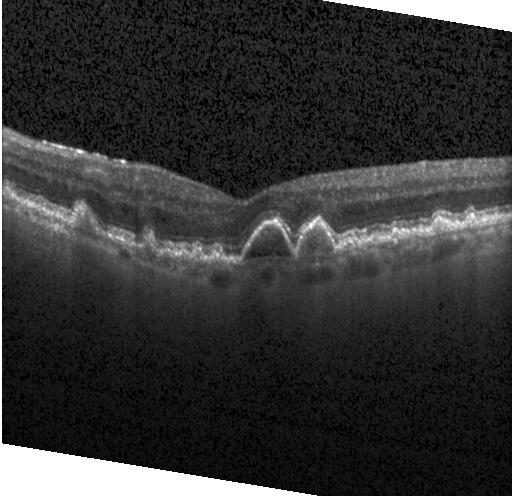 Acquired on a Heidelberg Spectralis; retinal OCT B-scan — Dx: drusen.